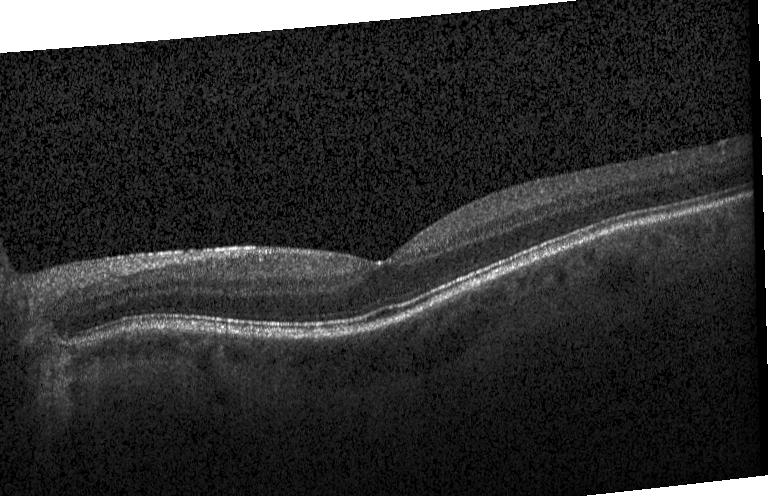

Optical coherence tomography scan
The scan shows no CNV, DME, or drusen.